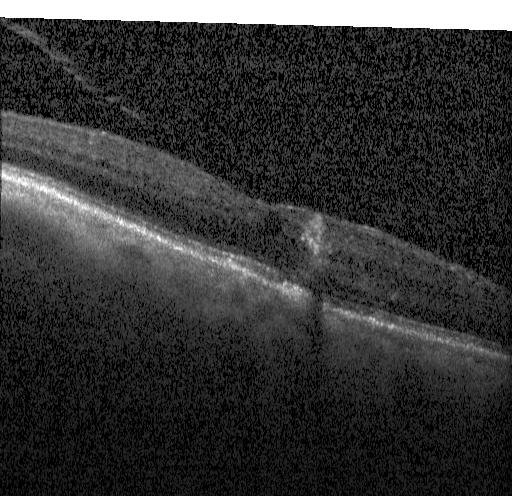

OCT scan showing DME.